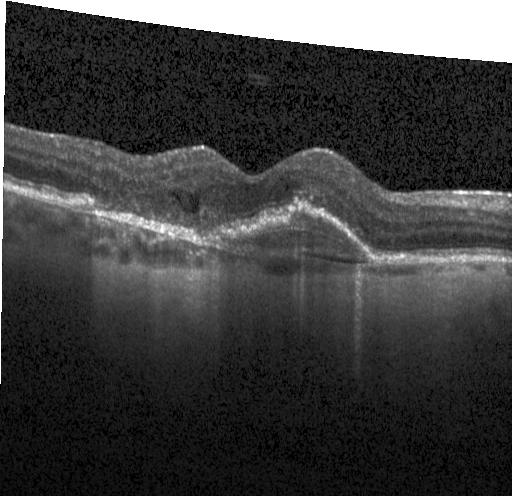

Spectral-domain OCT. Retinal OCT cross-section. Centered on the fovea. Acquired on a Heidelberg Spectralis. Finding: choroidal neovascularization.